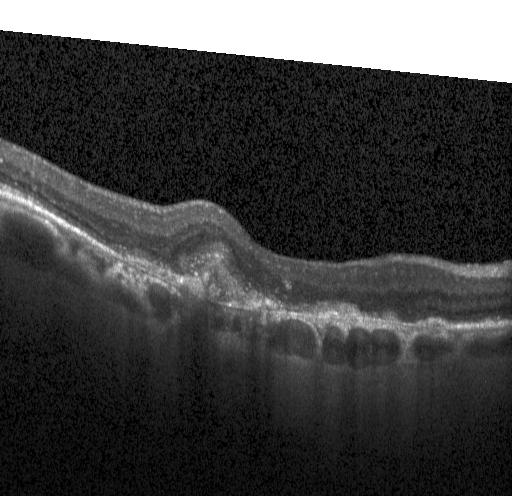
OCT B-scan. Spectral-domain optical coherence tomography.
The scan shows choroidal neovascularization.